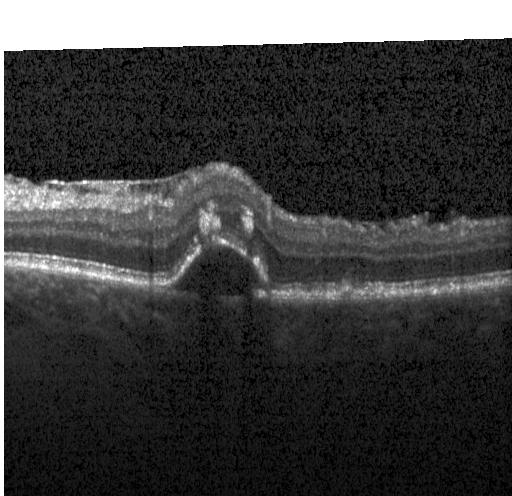

Choroidal neovascularization (CNV).